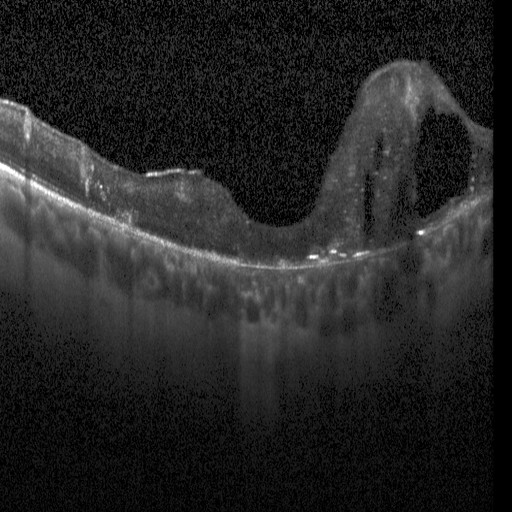 Optical coherence tomography B-scan
Assessment: diabetic macular edema (DME).